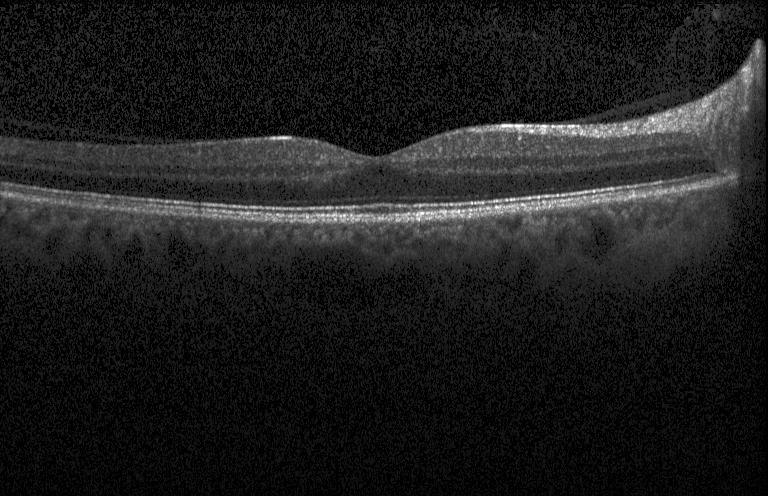
OCT scan showing no choroidal neovascularization, diabetic macular edema, or drusen.